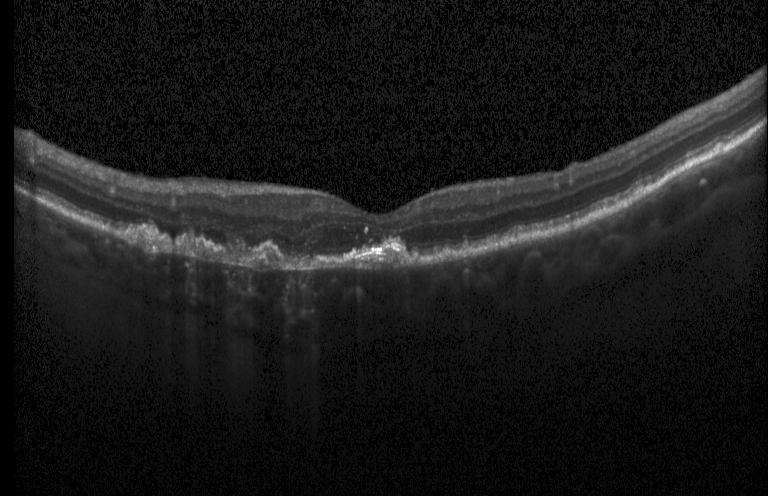

The scan shows choroidal neovascularization.